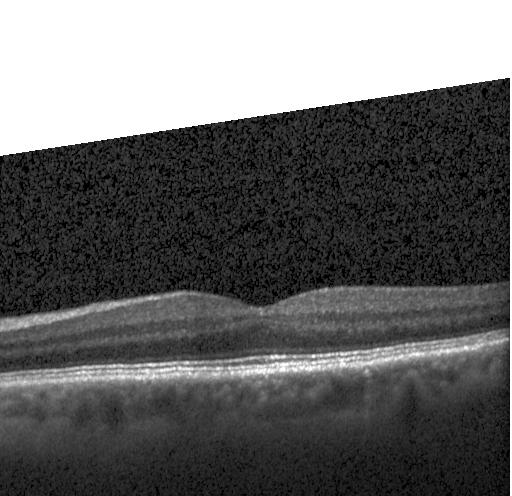 Optical coherence tomography B-scan; spectral-domain optical coherence tomography; Heidelberg Spectralis OCT system; horizontal scan through the fovea — Assessment: no choroidal neovascularization, diabetic macular edema, or drusen.